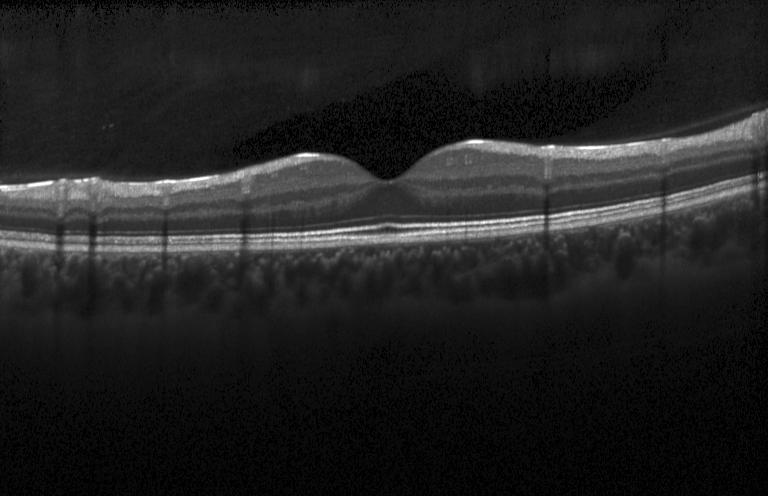
Dx: neither choroidal neovascularization, diabetic macular edema, nor drusen.